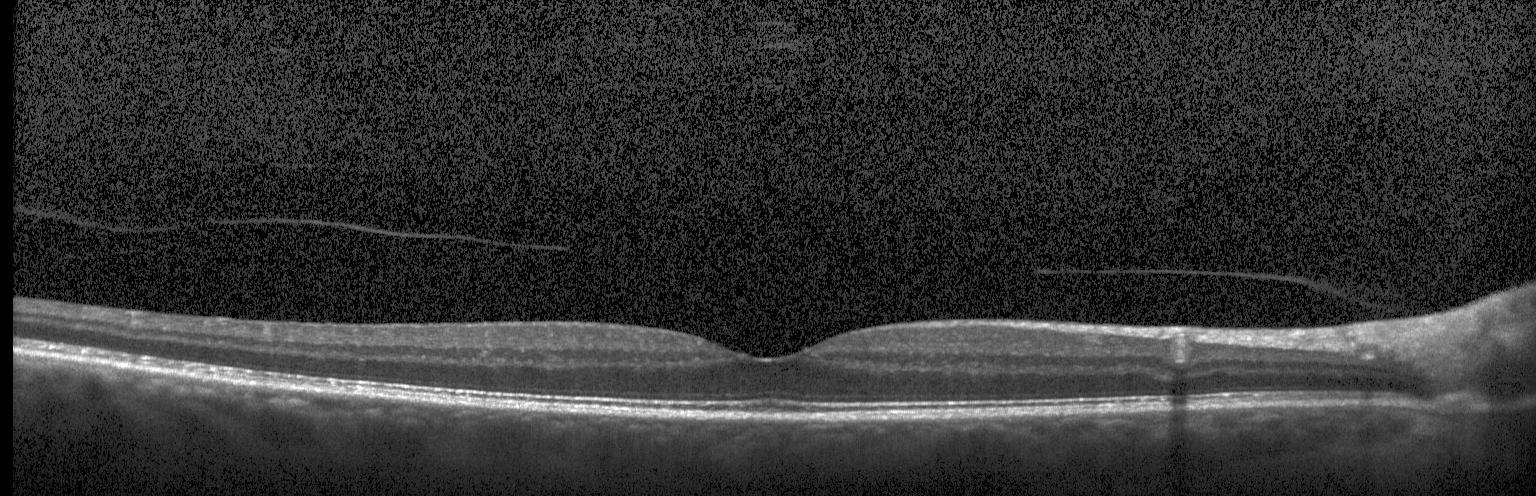

Spectral-domain optical coherence tomography; retinal OCT cross-section — Impression: neither choroidal neovascularization, diabetic macular edema, nor drusen.